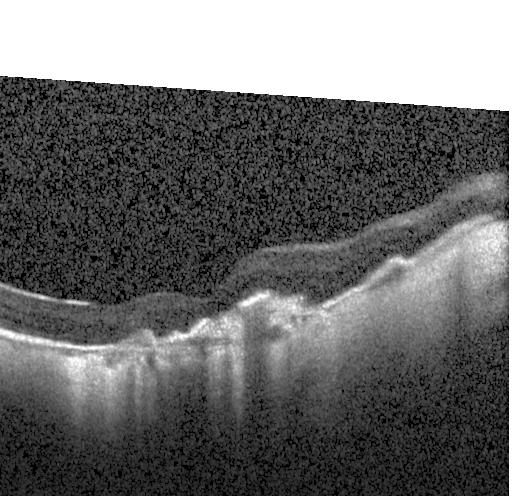

Centered on the fovea, spectral-domain optical coherence tomography, OCT B-scan. Assessment: choroidal neovascularization.